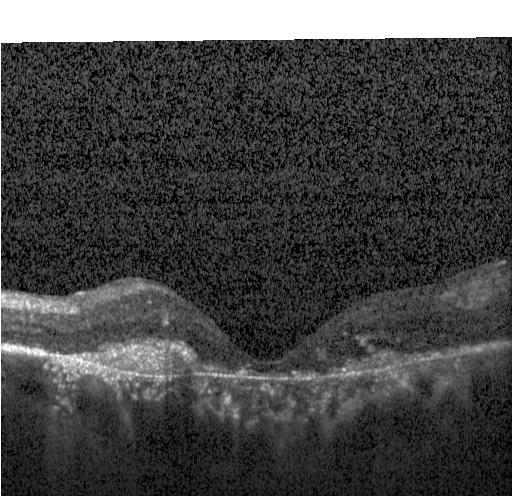
Retinal OCT B-scan · instrument: Heidelberg Spectralis · macular scan. Diagnosis: a choroidal neovascular membrane.